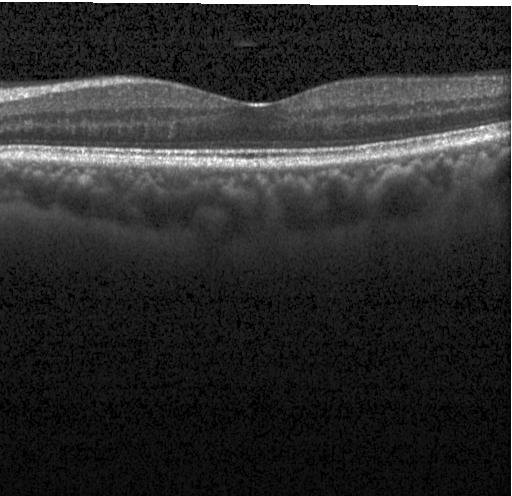
Retinal OCT cross-section. Acquired on a Heidelberg Spectralis — Impression: no CNV, no DME, and no drusen.